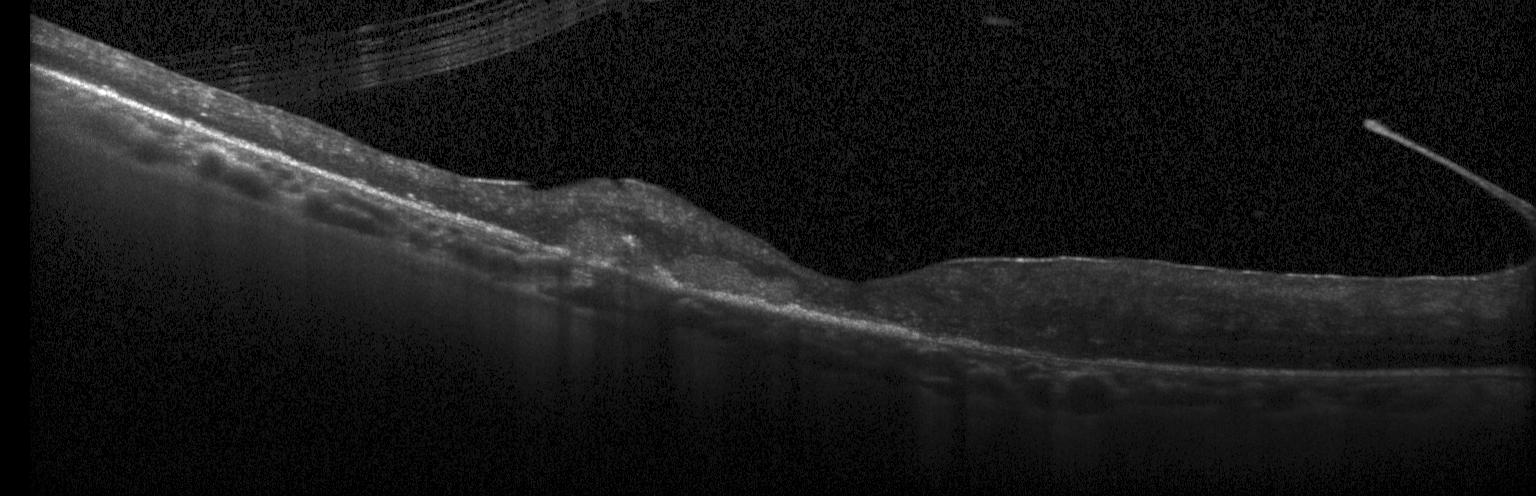 Finding: a choroidal neovascular membrane.